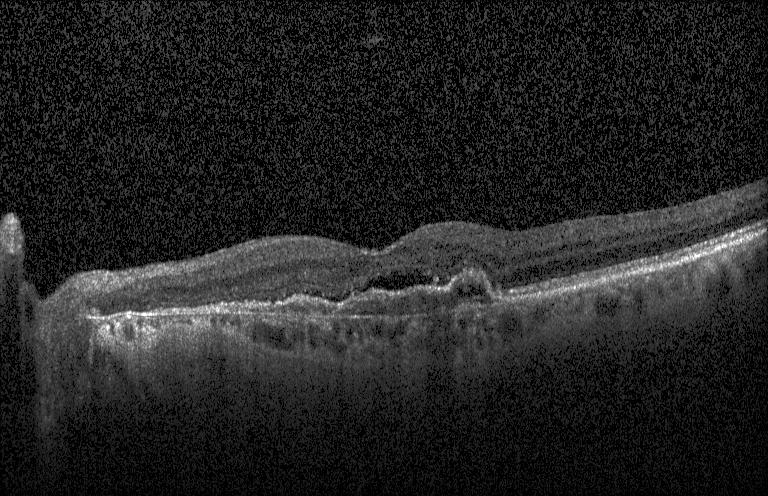

Diagnosis: a choroidal neovascular membrane.